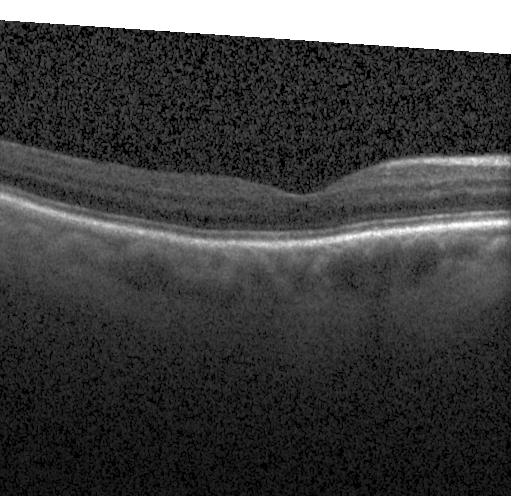
Optical coherence tomography B-scan · acquired on a Heidelberg Spectralis · spectral-domain OCT
OCT finding: no CNV, DME, or drusen.